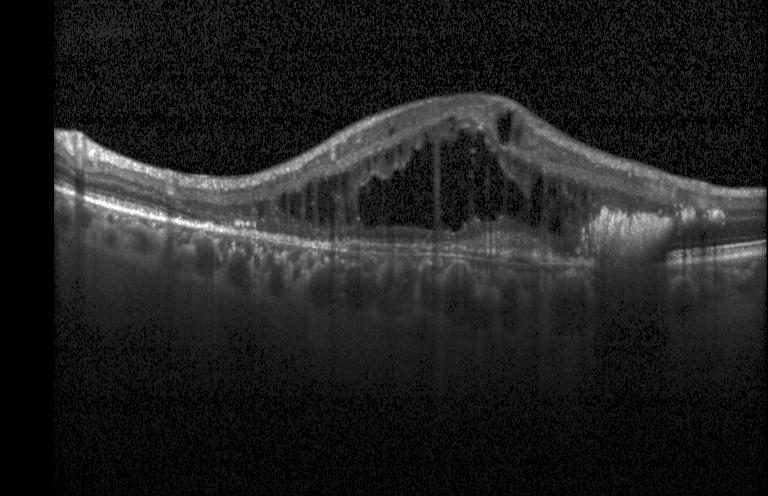 OCT line scan, macular scan, instrument: Heidelberg Spectralis, spectral-domain optical coherence tomography. This B-scan demonstrates a choroidal neovascular membrane.